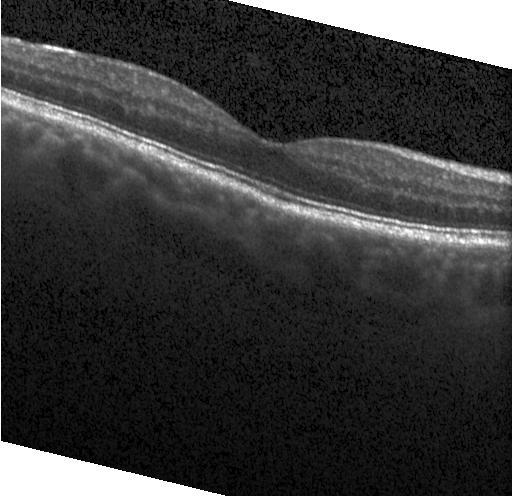 Optical coherence tomography scan, spectral-domain optical coherence tomography, Heidelberg Spectralis OCT system, horizontal scan through the fovea
This B-scan demonstrates no CNV, no DME, and no drusen.